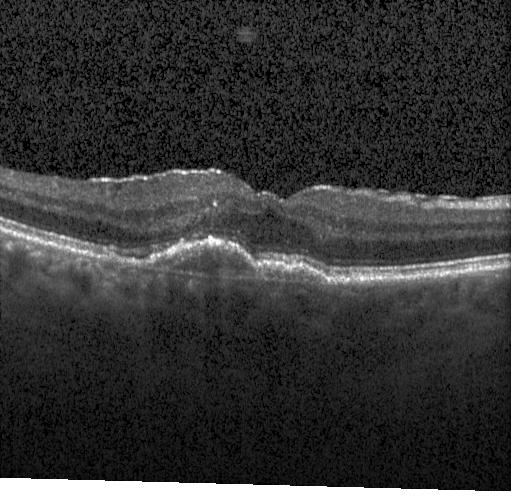

OCT B-scan showing CNV.